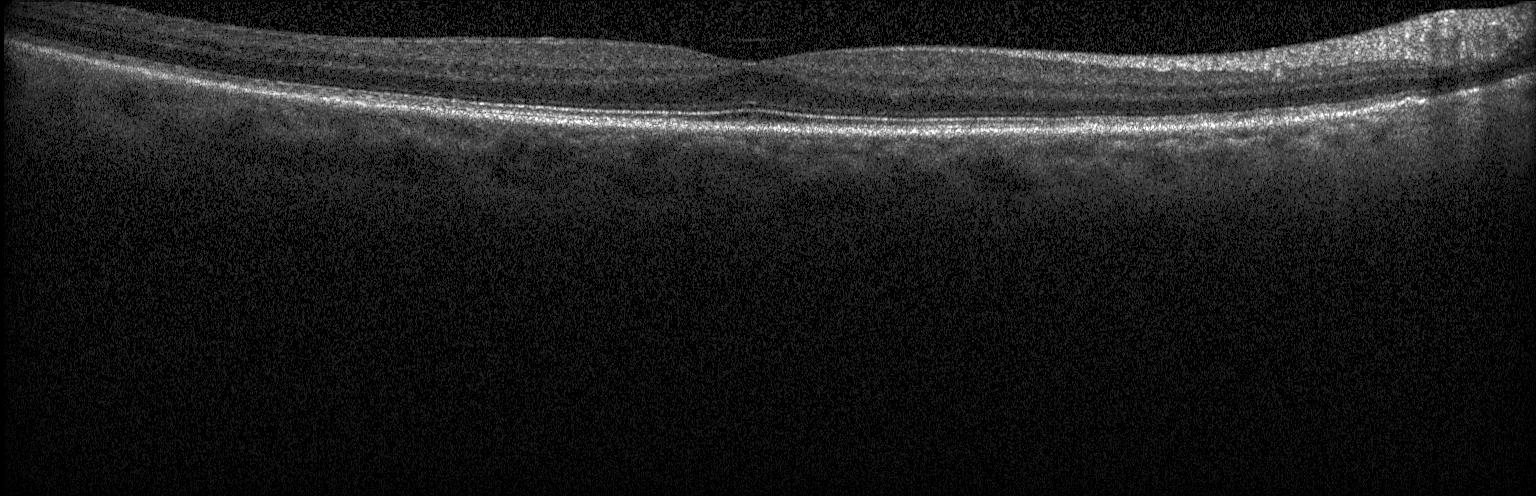
Spectral-domain OCT; retinal OCT cross-section.
Impression: neither CNV, DME, nor drusen.